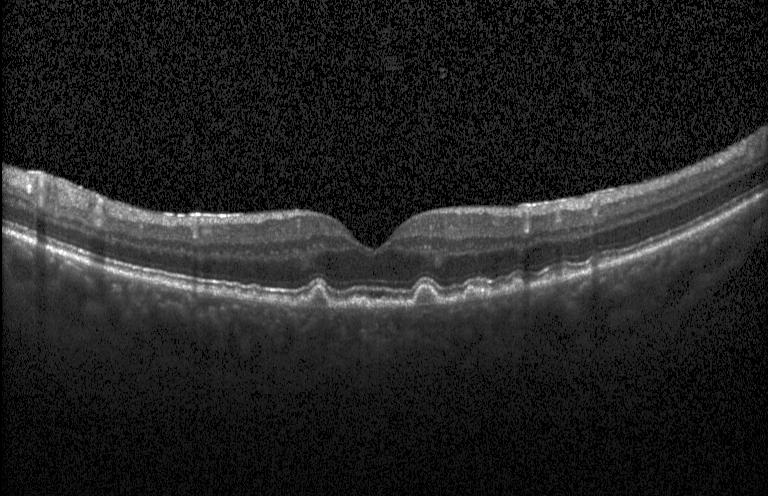

OCT B-scan showing multiple drusen.